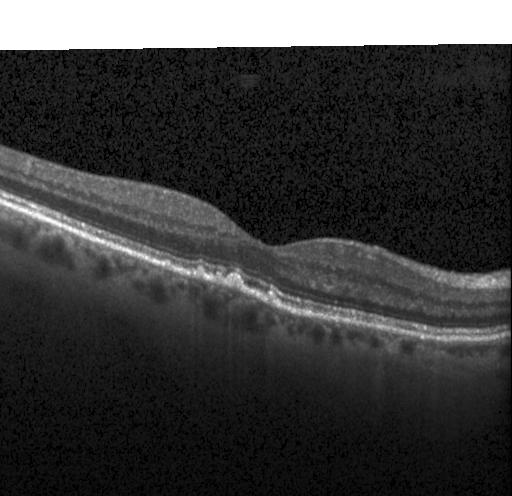 The scan shows sub-RPE drusenoid deposits.